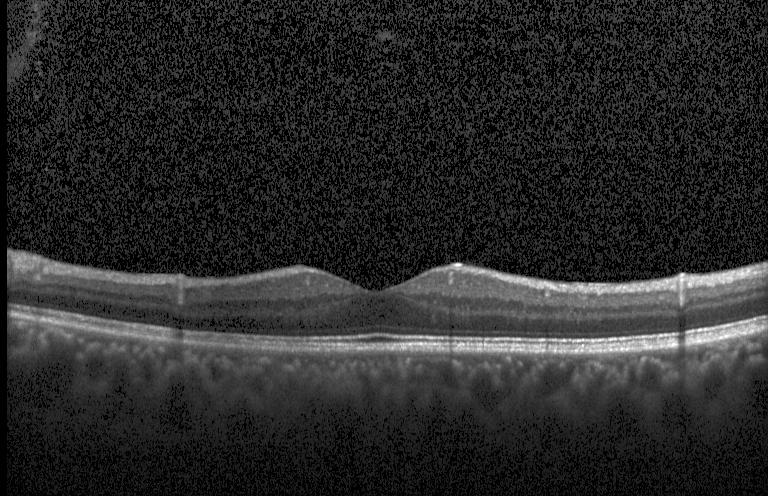 SD-OCT. Optical coherence tomography B-scan. Diagnosis: no CNV, DME, or drusen.